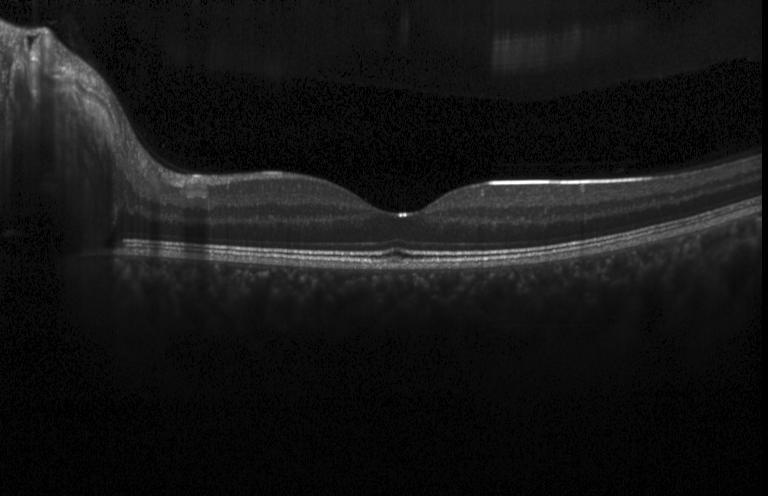
OCT finding: no choroidal neovascularization, no diabetic macular edema, and no drusen.